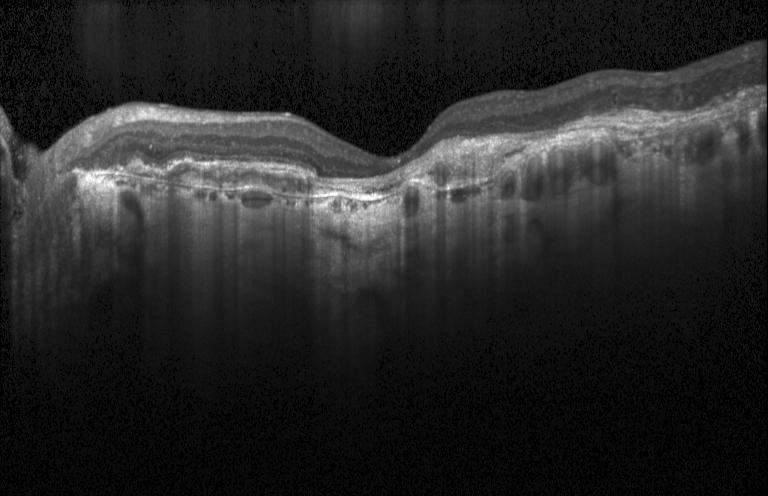
Retinal OCT B-scan.
This B-scan demonstrates choroidal neovascularization (CNV).